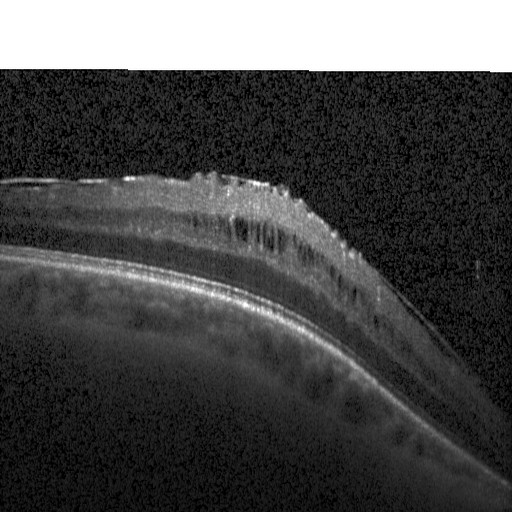 Optical coherence tomography B-scan. Macular scan. Instrument: Heidelberg Spectralis
Diabetic macular edema.